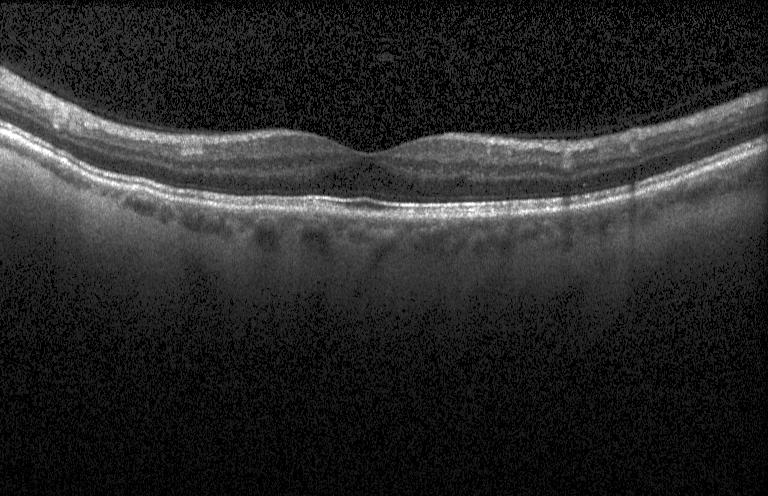

OCT B-scan; horizontal scan through the fovea — No CNV, no DME, and no drusen.